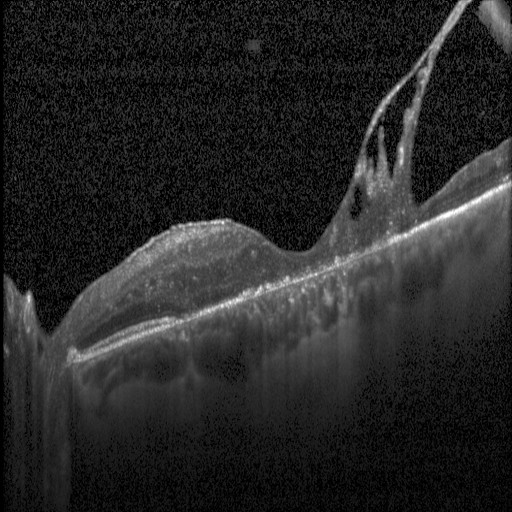
Spectral-domain optical coherence tomography, Heidelberg Spectralis OCT system, retinal OCT B-scan, fovea-centered. Finding: diabetic macular edema.